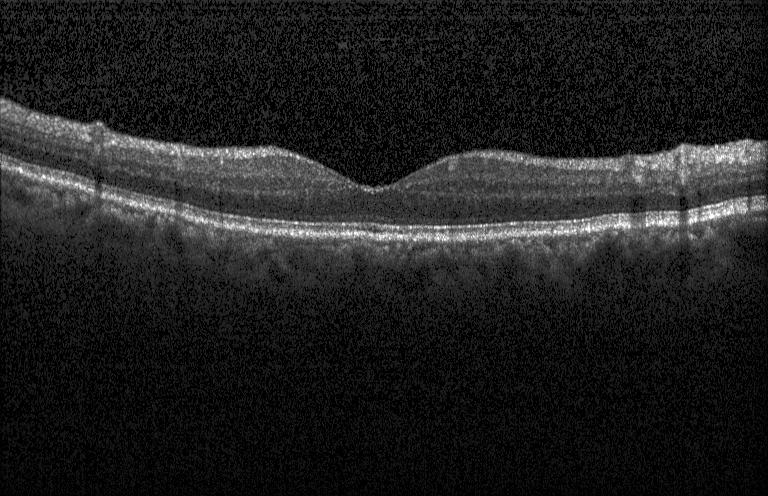 The scan shows no choroidal neovascularization, no diabetic macular edema, and no drusen.